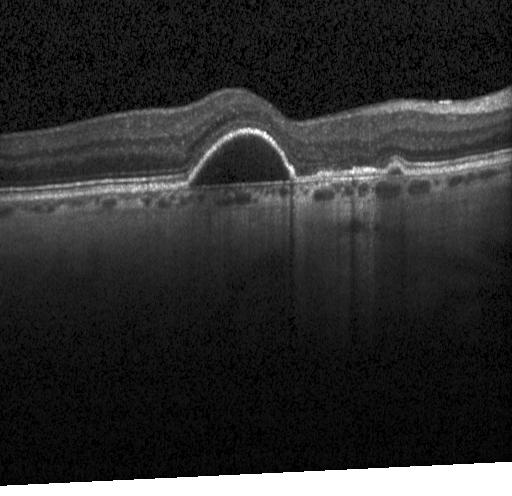 Retinal OCT cross-section, through the macula, Heidelberg Spectralis.
Diagnosis: choroidal neovascularization (CNV).